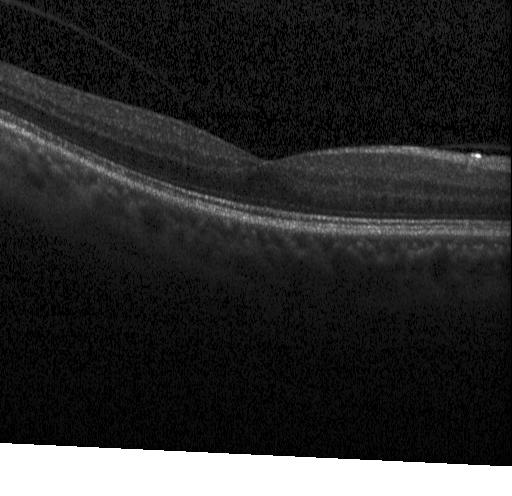
Centered on the fovea, retinal OCT cross-section, spectral-domain optical coherence tomography.
Impression: no evidence of CNV, DME, or drusen.